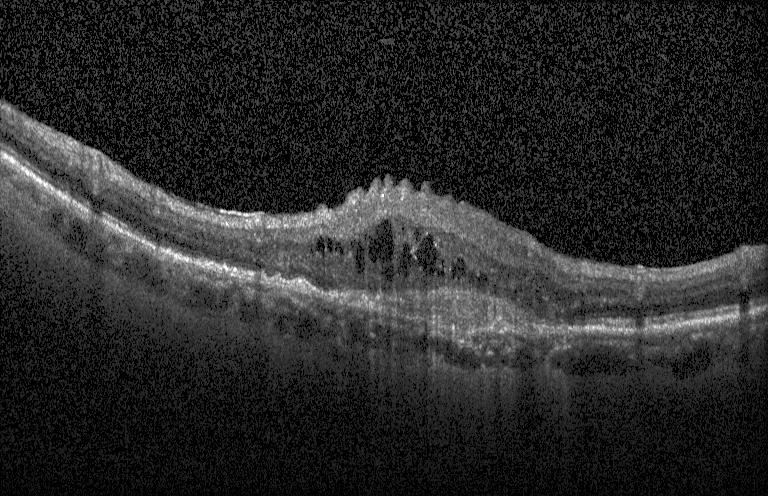

Retinal OCT B-scan
Choroidal neovascularization.